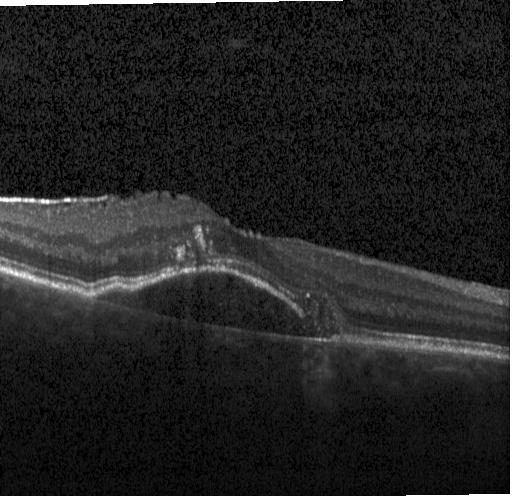
OCT scan showing choroidal neovascularization (CNV).